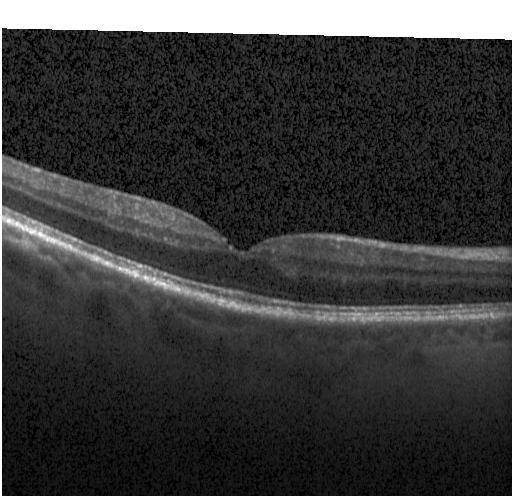
Retinal OCT cross-section, through the macula, instrument: Heidelberg Spectralis — Macular OCT: neither choroidal neovascularization, diabetic macular edema, nor drusen.